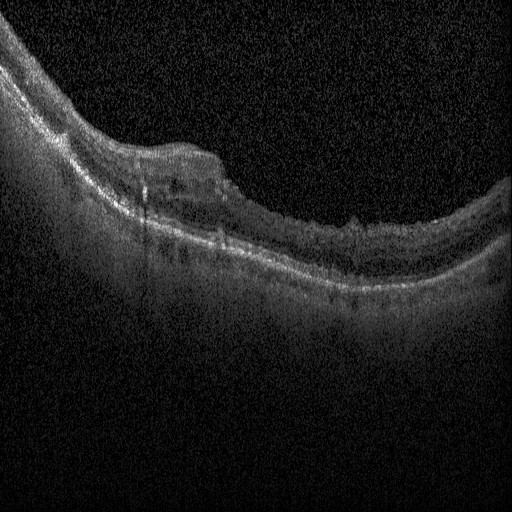
Diagnosis: diabetic macular edema (DME).